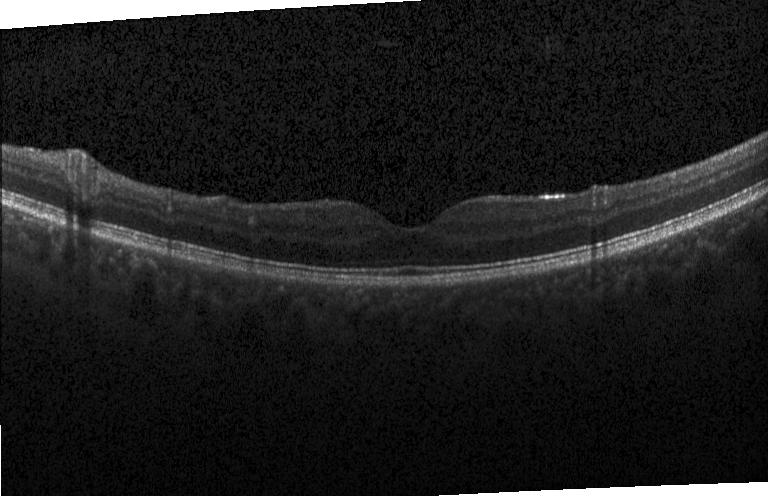

Optical coherence tomography scan. Spectral-domain OCT. OCT finding: no evidence of CNV, DME, or drusen.